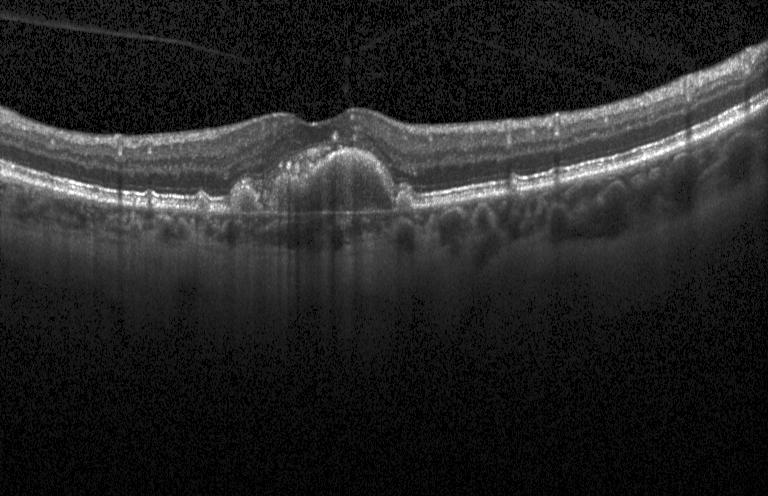
Optical coherence tomography scan · centered on the fovea · SD-OCT — Macular OCT: choroidal neovascularization.